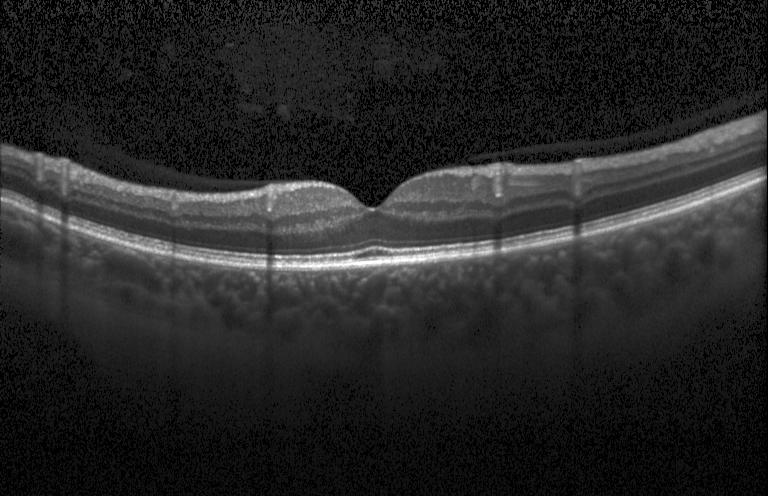

Acquired on a Heidelberg Spectralis. Macular scan. SD-OCT. Optical coherence tomography B-scan
Macular OCT: no CNV, DME, or drusen.